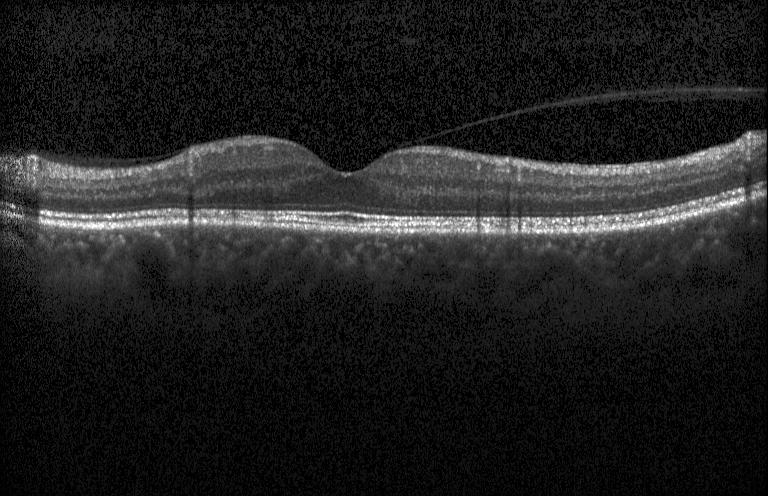
OCT line scan. Diagnosis: neither choroidal neovascularization, diabetic macular edema, nor drusen.